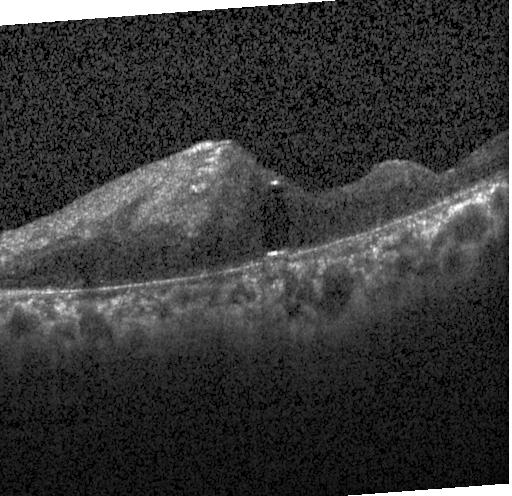
Macular scan, Heidelberg Spectralis OCT system, OCT B-scan.
Impression: a choroidal neovascular membrane.